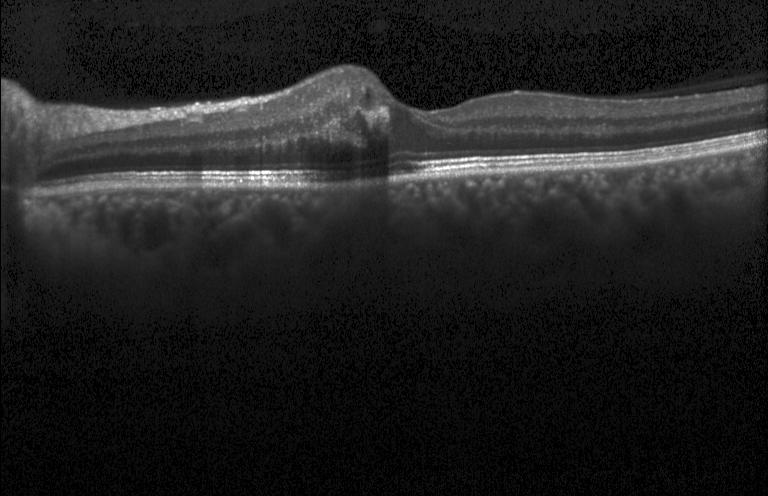
Heidelberg Spectralis OCT system; optical coherence tomography scan; spectral-domain optical coherence tomography; horizontal scan through the fovea
Impression: DME.